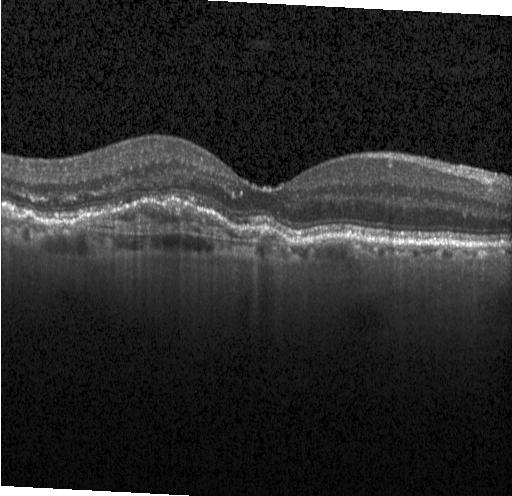
Retinal OCT B-scan, SD-OCT — Macular OCT: a choroidal neovascular membrane.